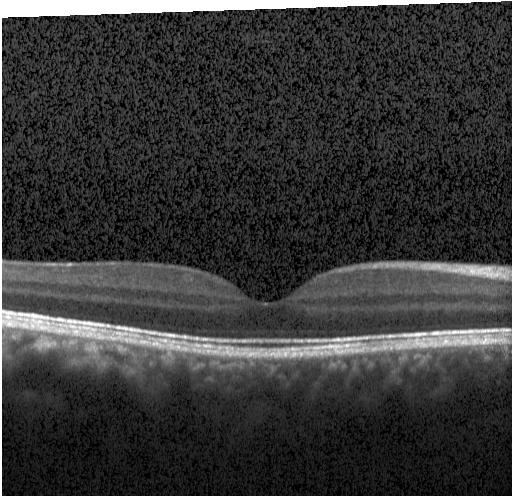

Spectral-domain OCT B-scan: no choroidal neovascularization, no diabetic macular edema, and no drusen.